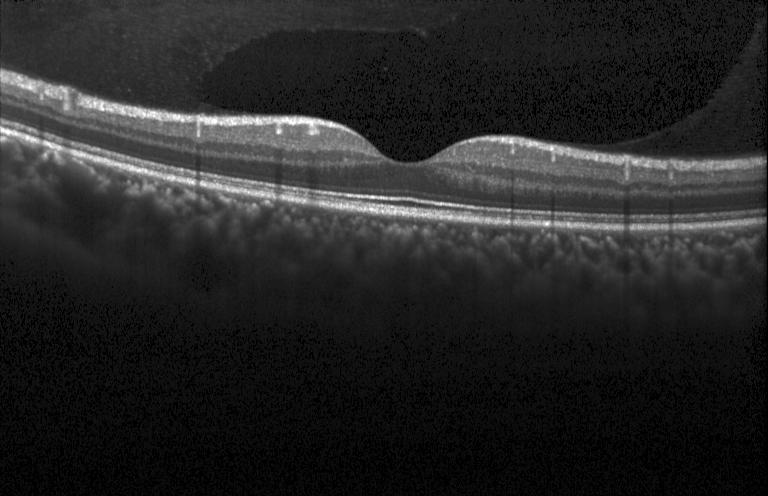

Retinal OCT B-scan; SD-OCT
Assessment: neither CNV, DME, nor drusen.